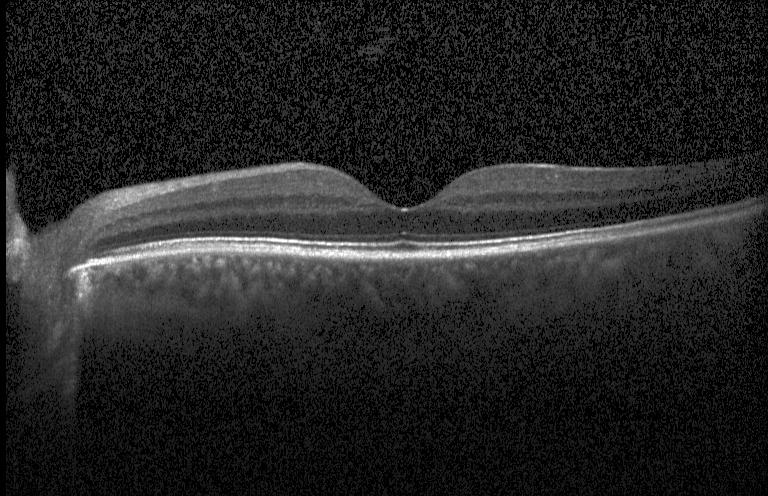
Spectral-domain OCT, optical coherence tomography B-scan, macular scan. Finding: no choroidal neovascularization, diabetic macular edema, or drusen.